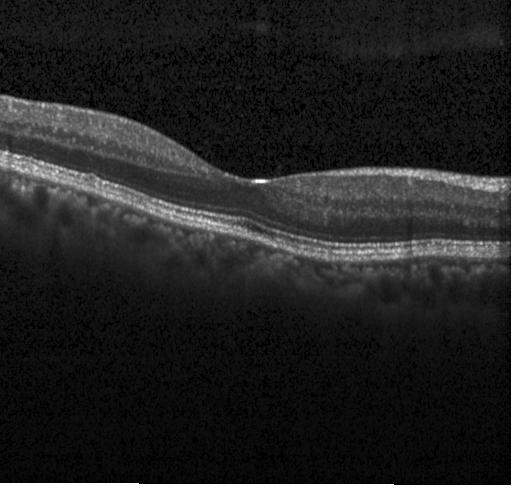 OCT B-scan showing no evidence of choroidal neovascularization, diabetic macular edema, or drusen.